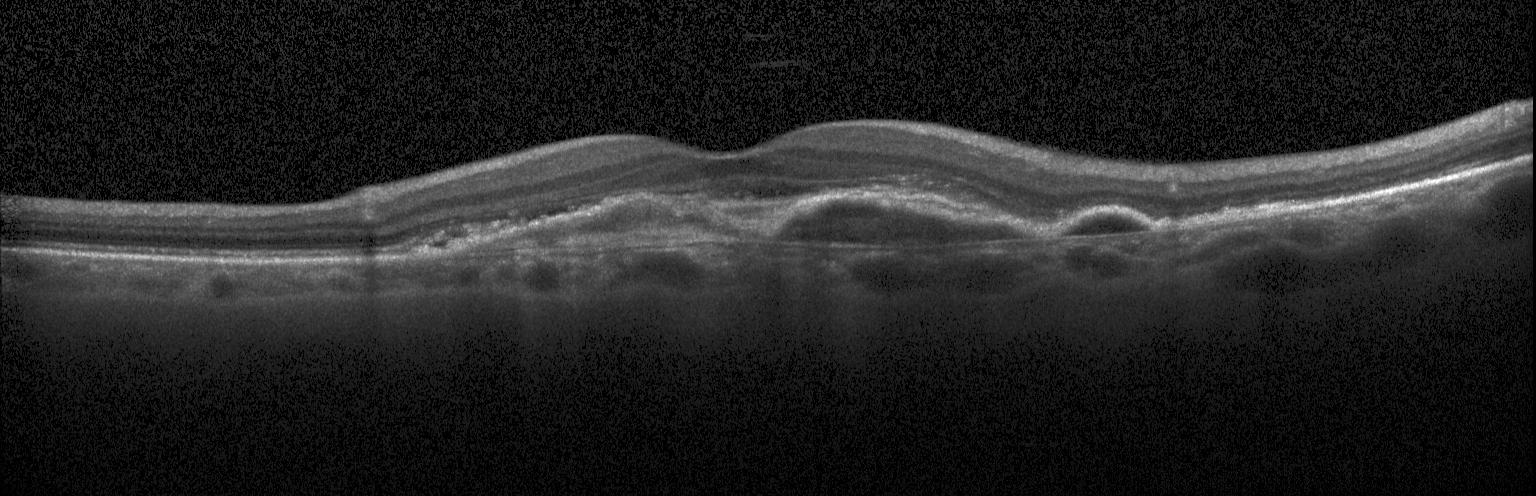 Instrument: Heidelberg Spectralis. Centered on the fovea. Spectral-domain OCT. Optical coherence tomography scan. Diagnosis: a choroidal neovascular membrane.